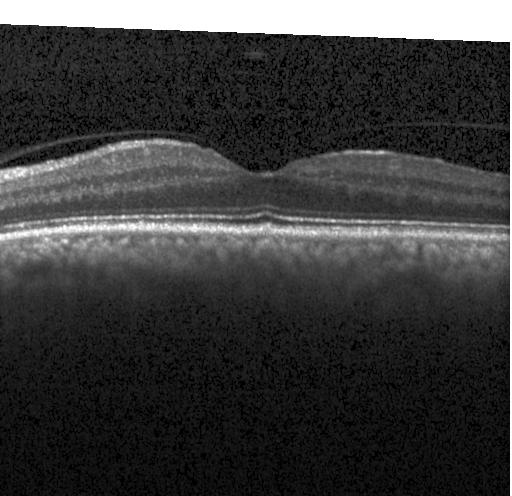 Optical coherence tomography B-scan. Diagnosis: no evidence of CNV, DME, or drusen.